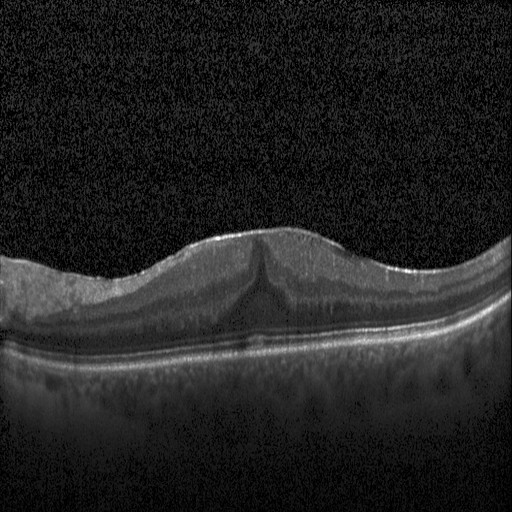 Optical coherence tomography B-scan. Centered on the fovea.
OCT finding: diabetic macular edema.